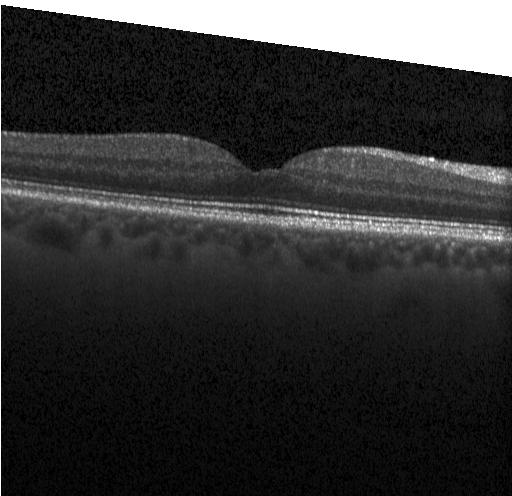
Acquired on a Heidelberg Spectralis; SD-OCT; OCT line scan; macular scan
Finding: no evidence of CNV, DME, or drusen.